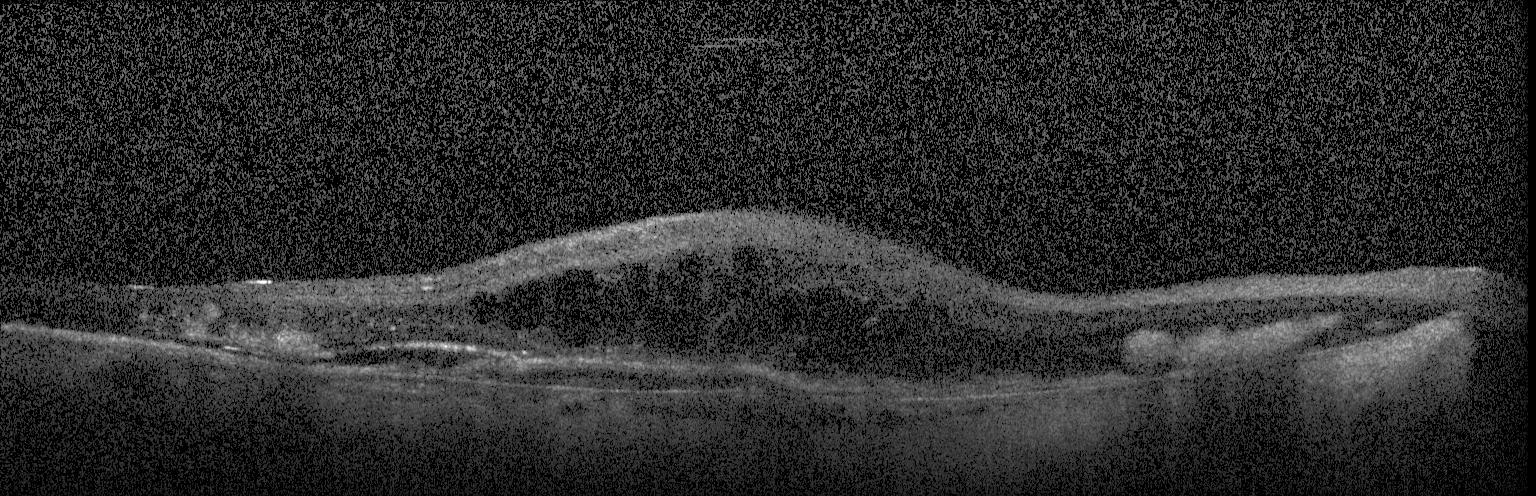

SD-OCT. Instrument: Heidelberg Spectralis. Optical coherence tomography scan. This B-scan demonstrates CNV.